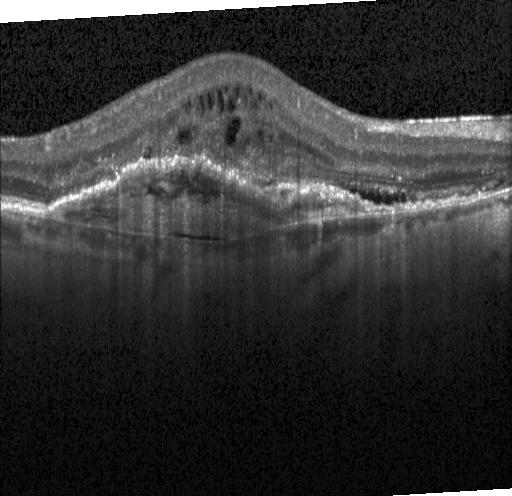 This B-scan demonstrates a choroidal neovascular membrane.